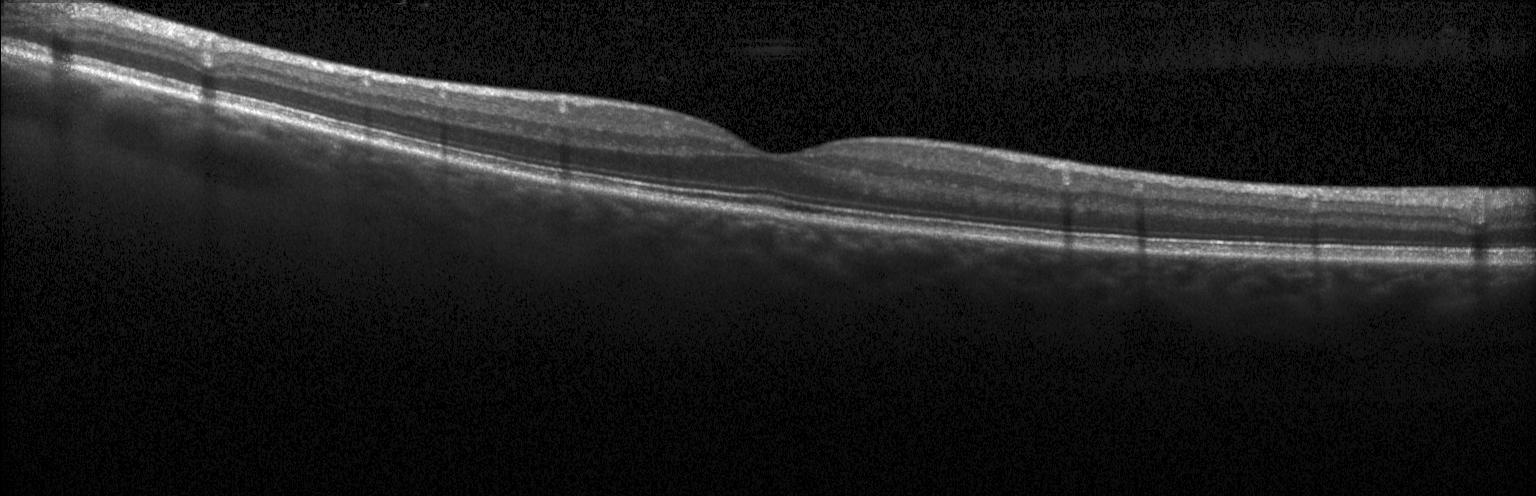
Instrument: Heidelberg Spectralis. OCT line scan. Macular scan.
Impression: no evidence of CNV, DME, or drusen.